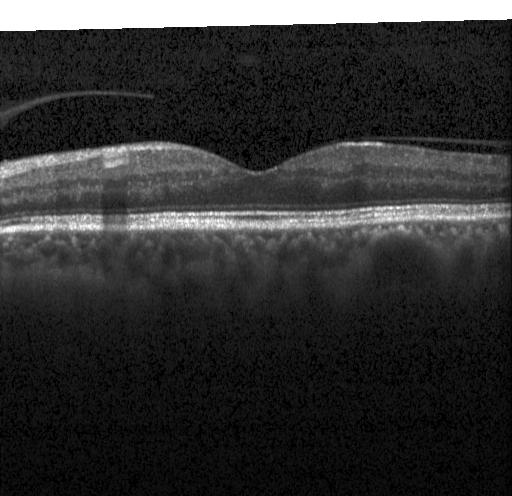

Retinal OCT B-scan, Heidelberg Spectralis. Macular OCT: no choroidal neovascularization, no diabetic macular edema, and no drusen.